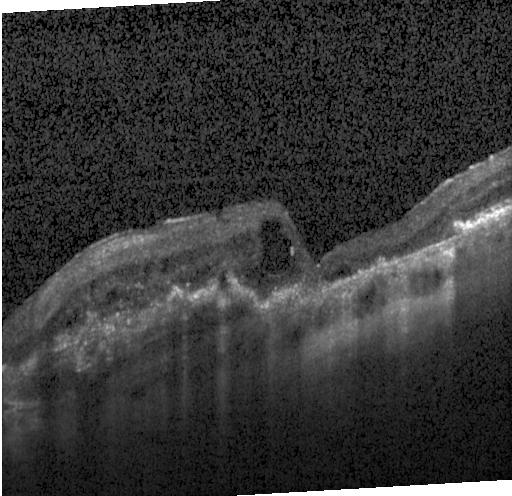

Impression: a choroidal neovascular membrane.